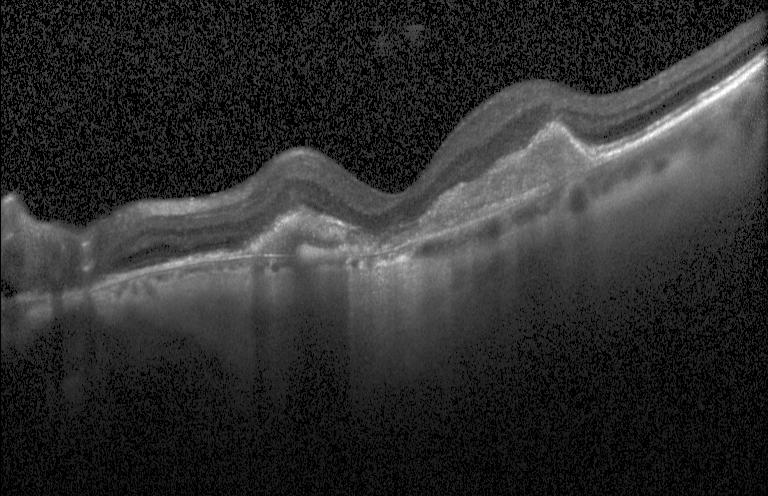 Macular scan, OCT line scan.
Dx: choroidal neovascularization (CNV).